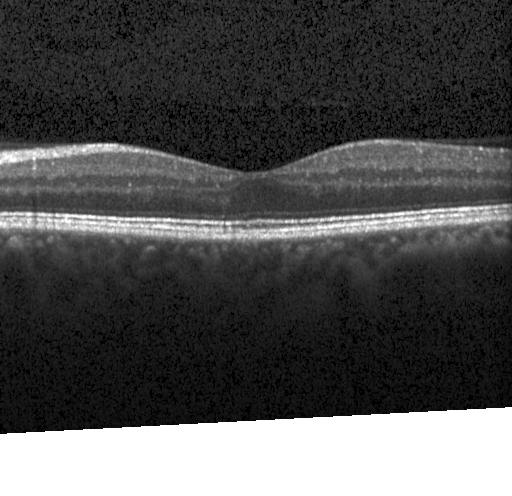

Diagnosis: neither CNV, DME, nor drusen.